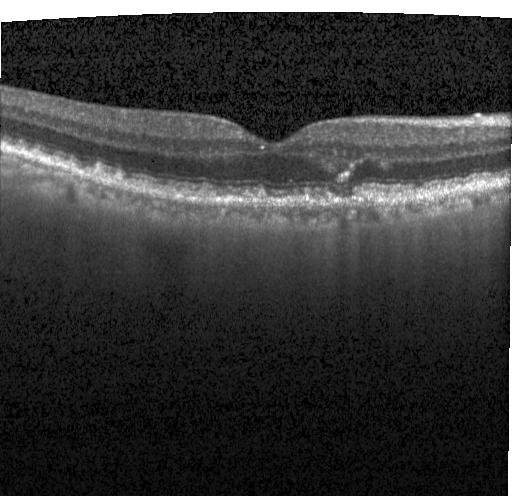
Impression: multiple drusen.